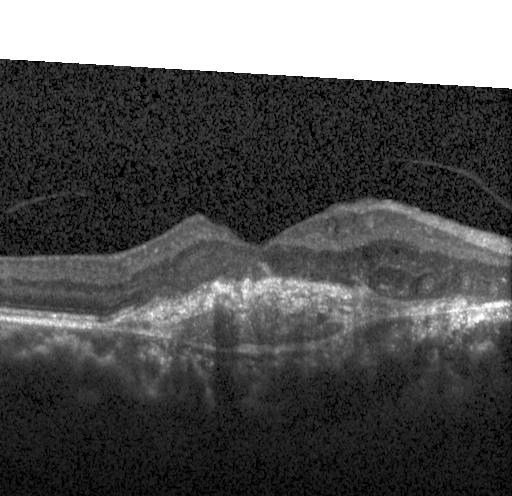

Horizontal scan through the fovea; retinal OCT B-scan — Impression: a choroidal neovascular membrane.